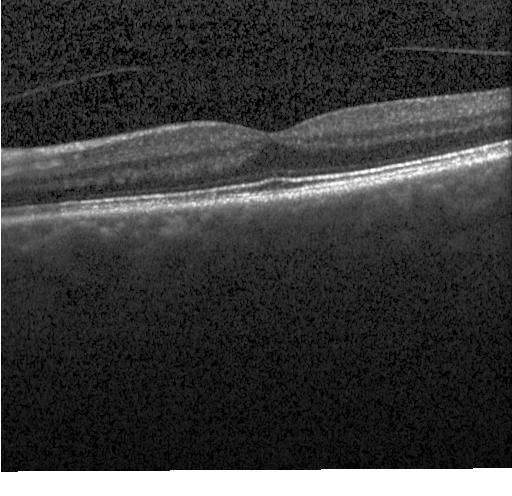 The scan shows no choroidal neovascularization, no diabetic macular edema, and no drusen.